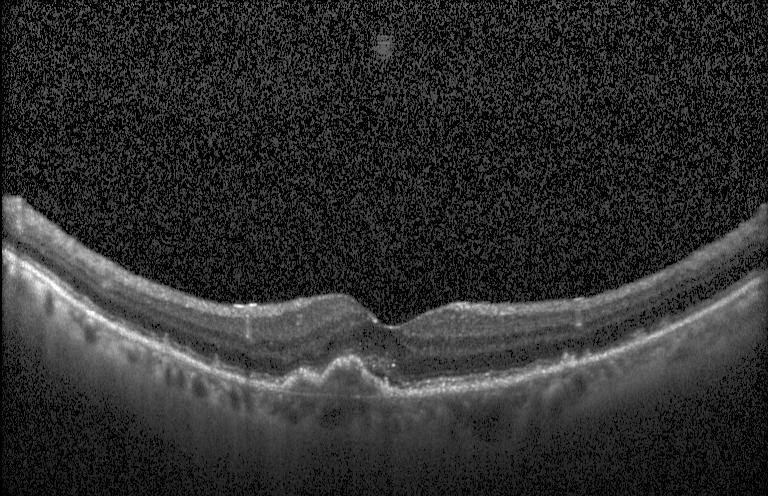 Macular scan · spectral-domain OCT · instrument: Heidelberg Spectralis · OCT line scan.
Dx: a choroidal neovascular membrane.